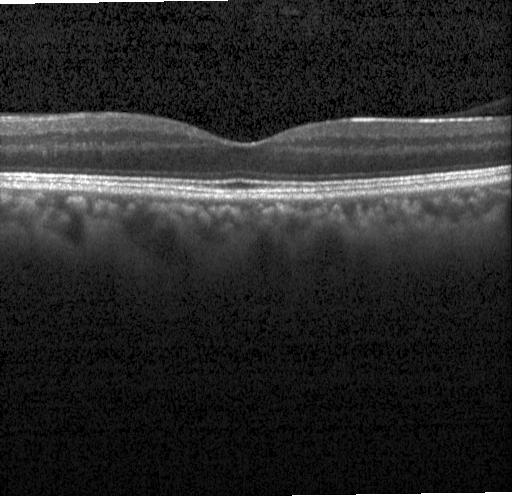
Through the macula; optical coherence tomography scan; instrument: Heidelberg Spectralis; spectral-domain OCT
This B-scan demonstrates neither CNV, DME, nor drusen.